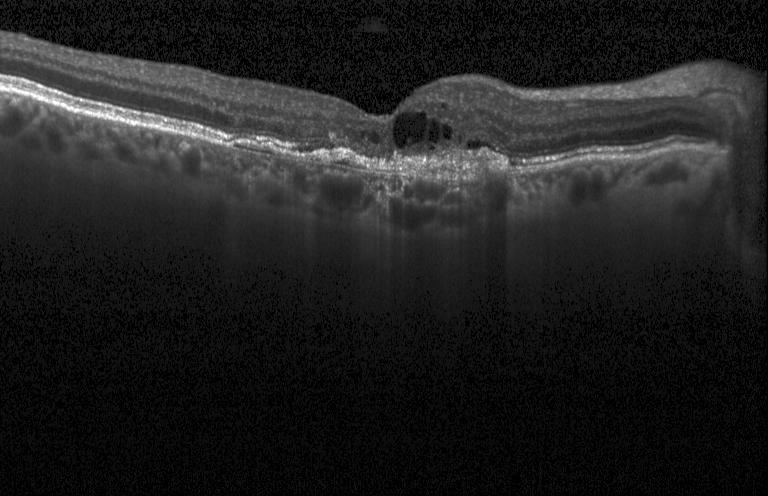

Heidelberg Spectralis OCT system, OCT line scan. Macular OCT: choroidal neovascularization (CNV).